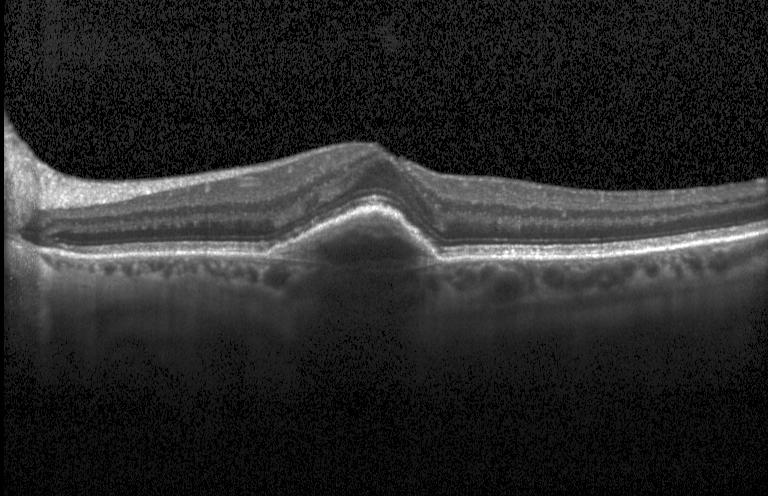

Heidelberg Spectralis OCT system, optical coherence tomography scan.
Diagnosis: a choroidal neovascular membrane.